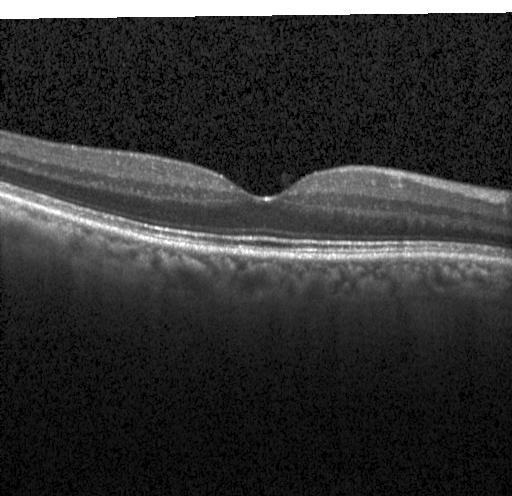
Impression: no CNV, no DME, and no drusen.